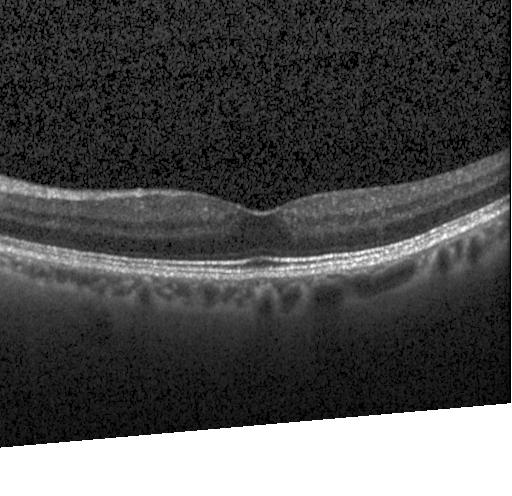

Dx: no evidence of CNV, DME, or drusen.